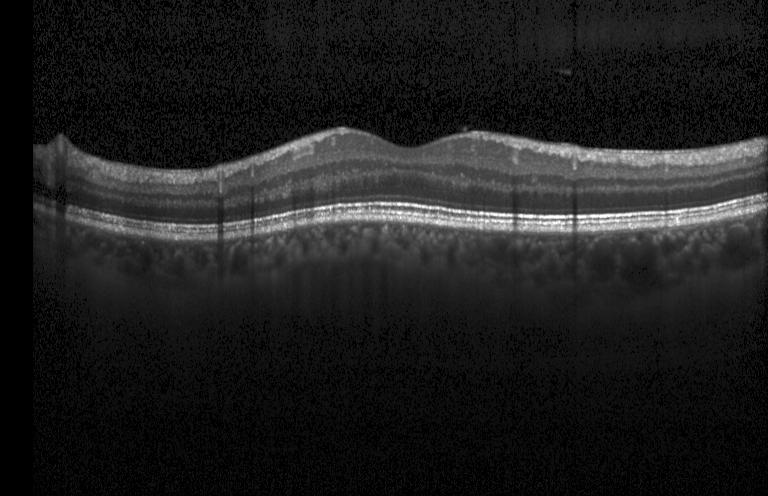 Retinal OCT B-scan, spectral-domain optical coherence tomography, acquired on a Heidelberg Spectralis — Impression: neither choroidal neovascularization, diabetic macular edema, nor drusen.